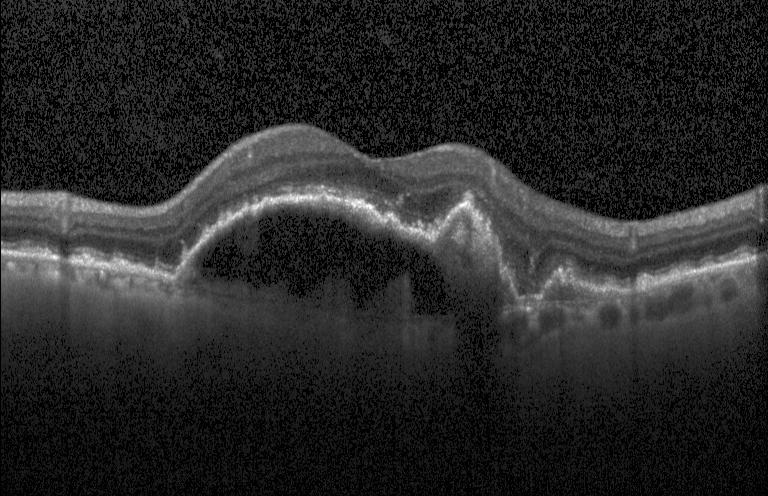

Spectral-domain OCT. OCT line scan. Instrument: Heidelberg Spectralis.
The scan shows choroidal neovascularization (CNV).